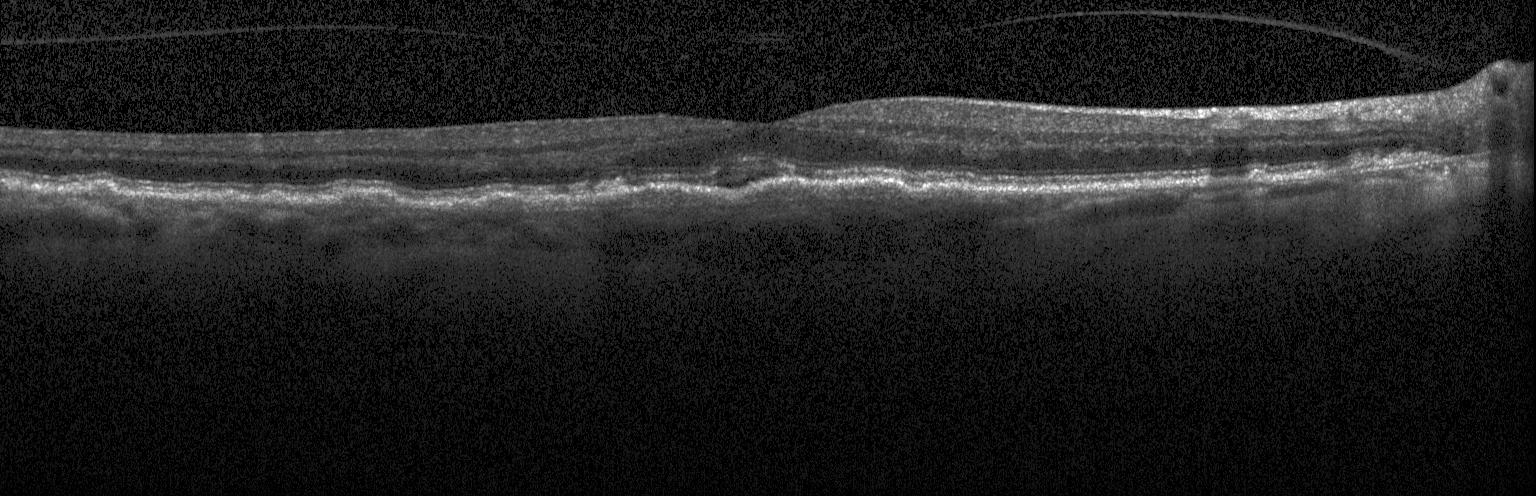
Dx: a choroidal neovascular membrane.